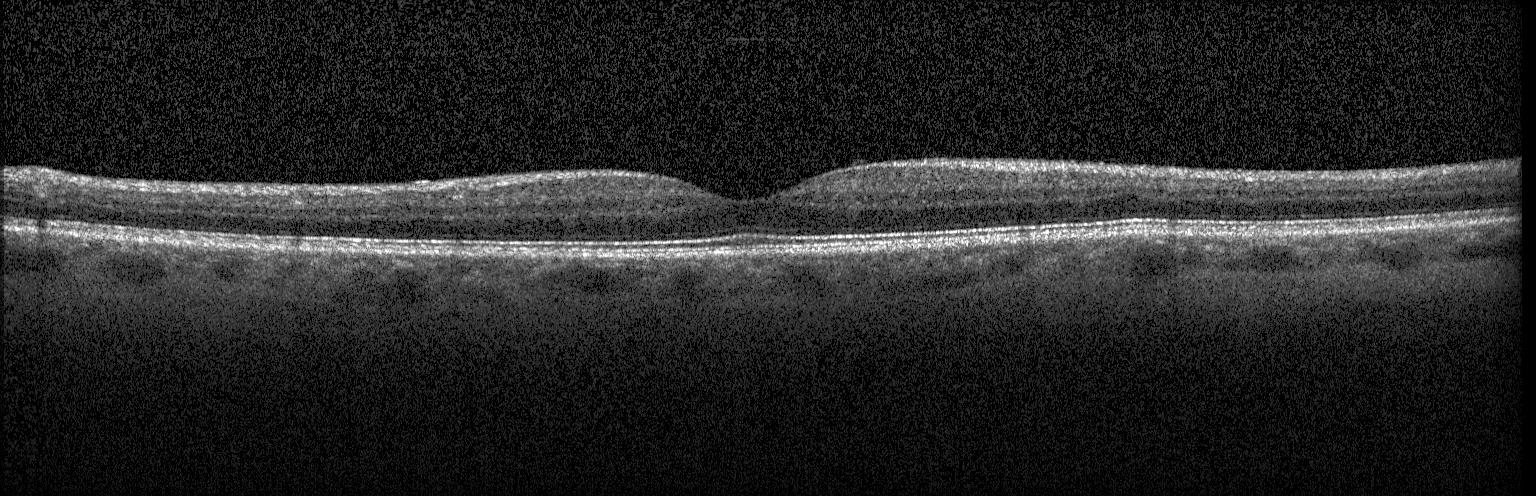 Dx: no CNV, DME, or drusen.